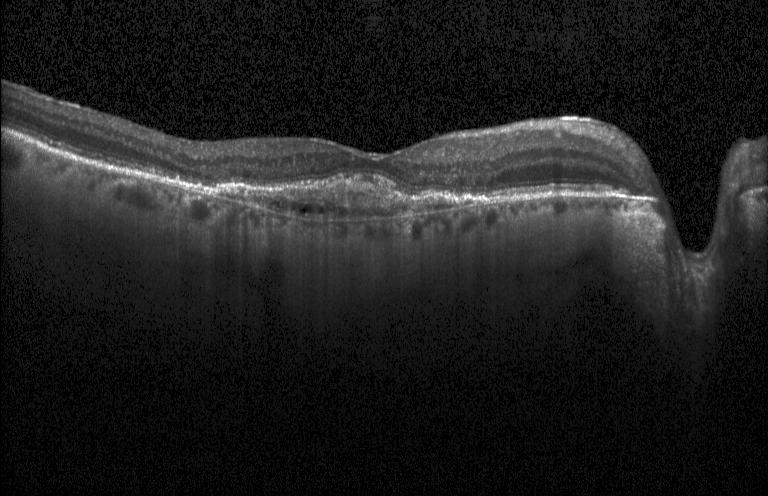 A choroidal neovascular membrane.